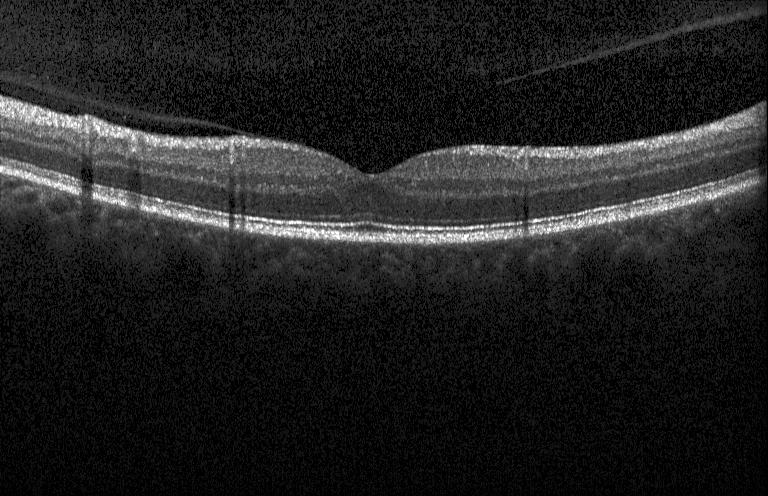 SD-OCT. OCT B-scan. Horizontal scan through the fovea.
Finding: no choroidal neovascularization, no diabetic macular edema, and no drusen.